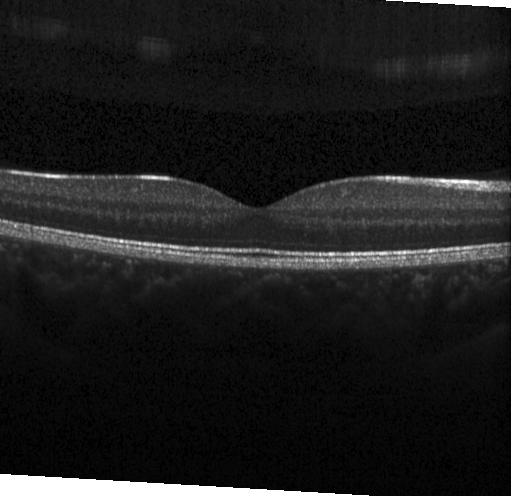 Heidelberg Spectralis · retinal OCT cross-section
Assessment: no CNV, DME, or drusen.